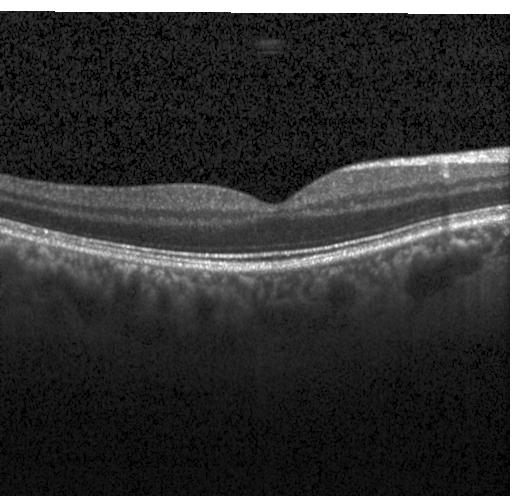 OCT B-scan, macular scan
Diagnosis: no choroidal neovascularization, diabetic macular edema, or drusen.